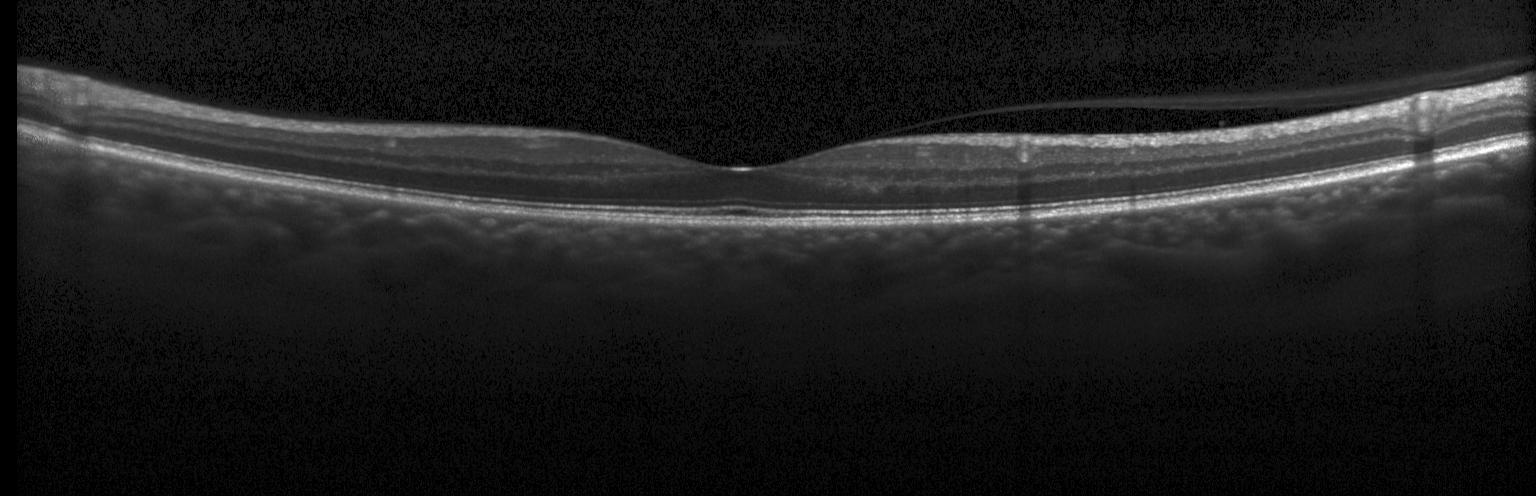

Retinal OCT B-scan — Macular OCT: no CNV, DME, or drusen.